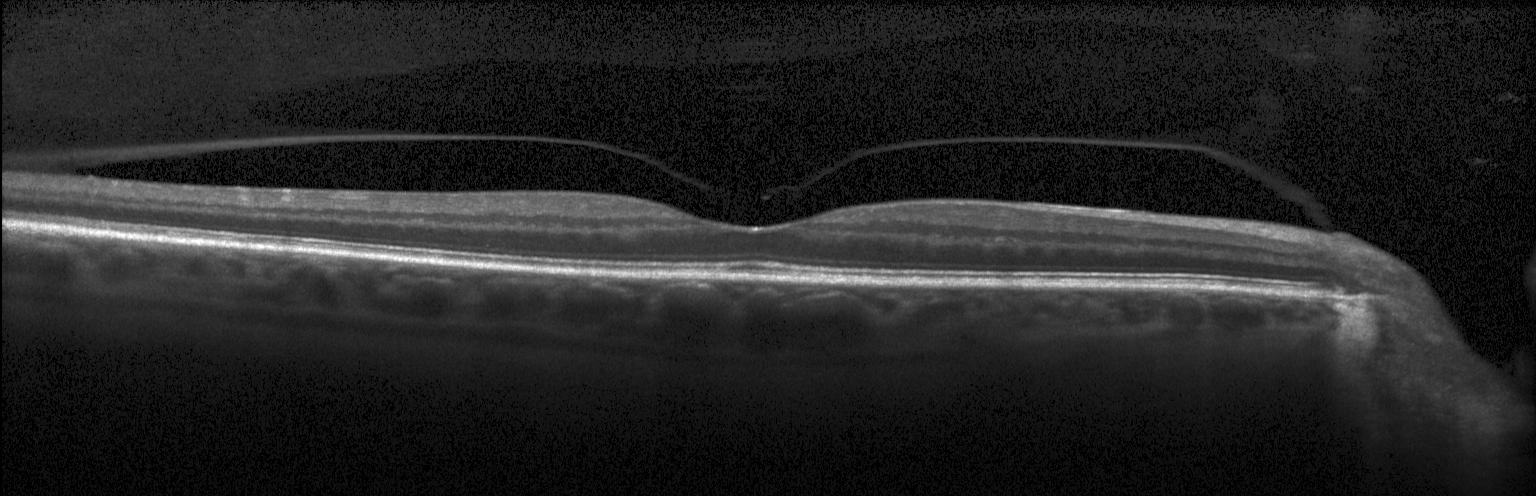

Optical coherence tomography scan · Heidelberg Spectralis · horizontal scan through the fovea — Macular OCT: no CNV, no DME, and no drusen.